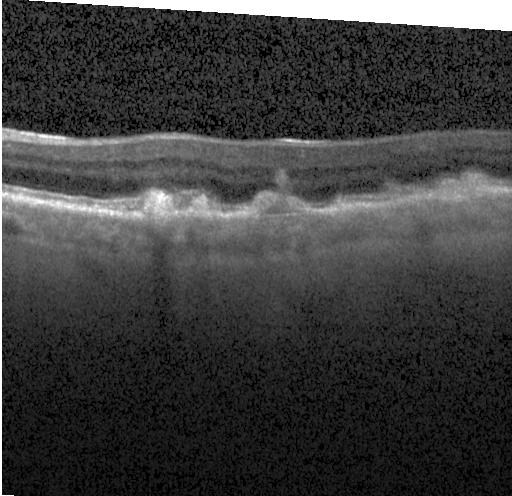

Horizontal scan through the fovea · retinal OCT B-scan · acquired on a Heidelberg Spectralis · spectral-domain OCT — Diagnosis: multiple drusen.